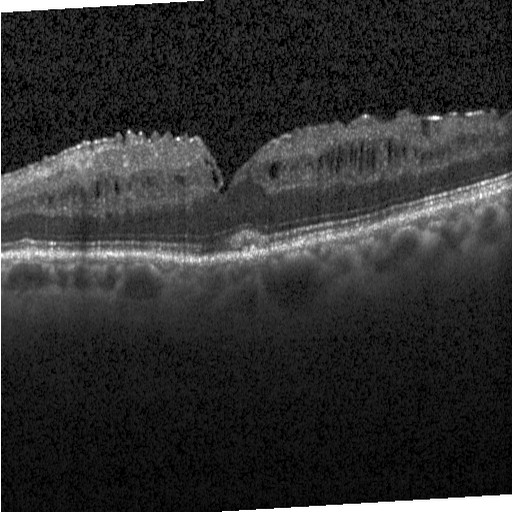
DME.